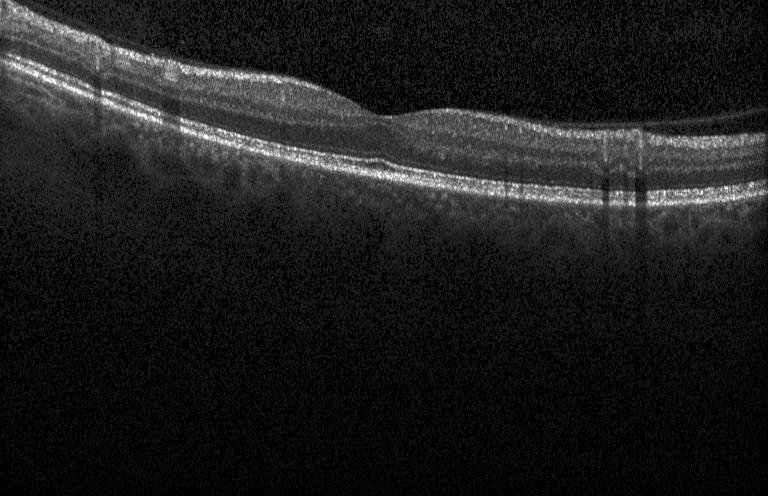 Horizontal scan through the fovea; OCT line scan; Heidelberg Spectralis OCT system. Finding: no evidence of CNV, DME, or drusen.